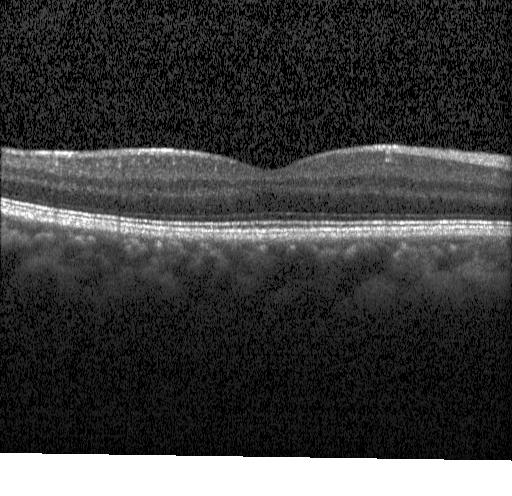
Diagnosis: no evidence of CNV, DME, or drusen.